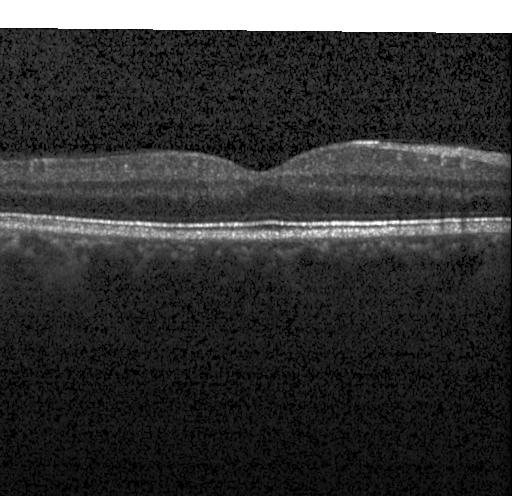

Horizontal scan through the fovea. Optical coherence tomography scan. Heidelberg Spectralis — No choroidal neovascularization, diabetic macular edema, or drusen.